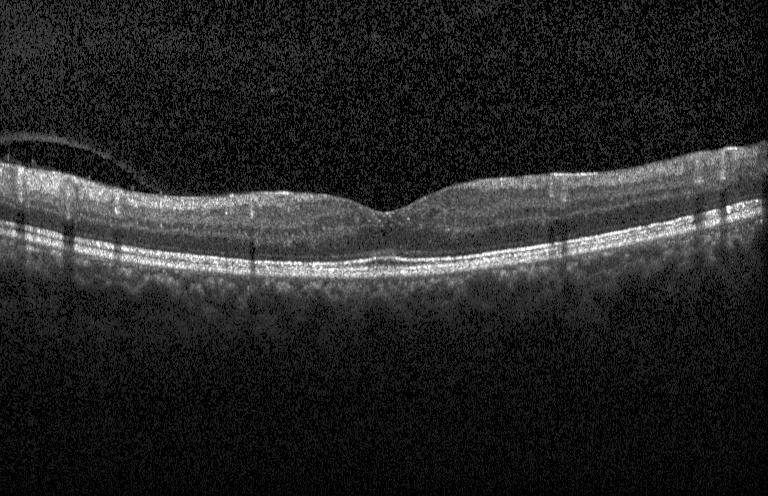 SD-OCT. OCT line scan.
Diagnosis: no CNV, DME, or drusen.